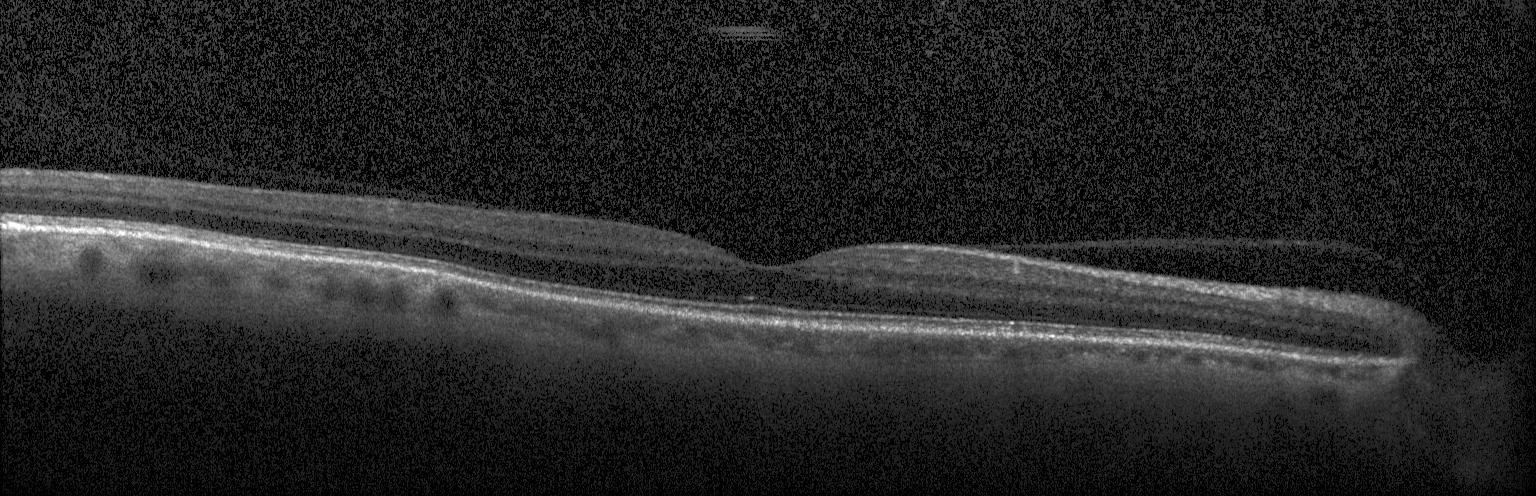 Spectral-domain optical coherence tomography, optical coherence tomography scan, Heidelberg Spectralis. Assessment: no evidence of CNV, DME, or drusen.